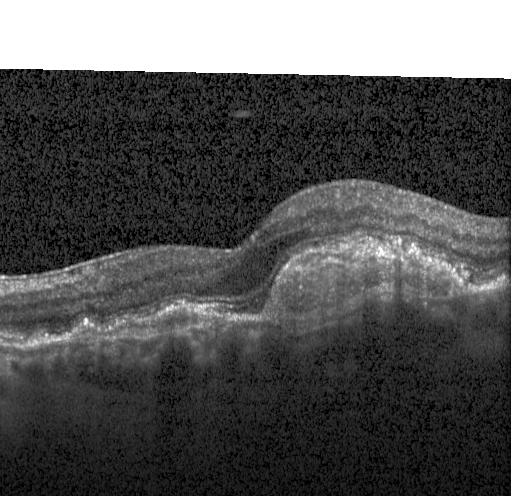

Optical coherence tomography B-scan, Heidelberg Spectralis, spectral-domain OCT
Diagnosis: choroidal neovascularization (CNV).